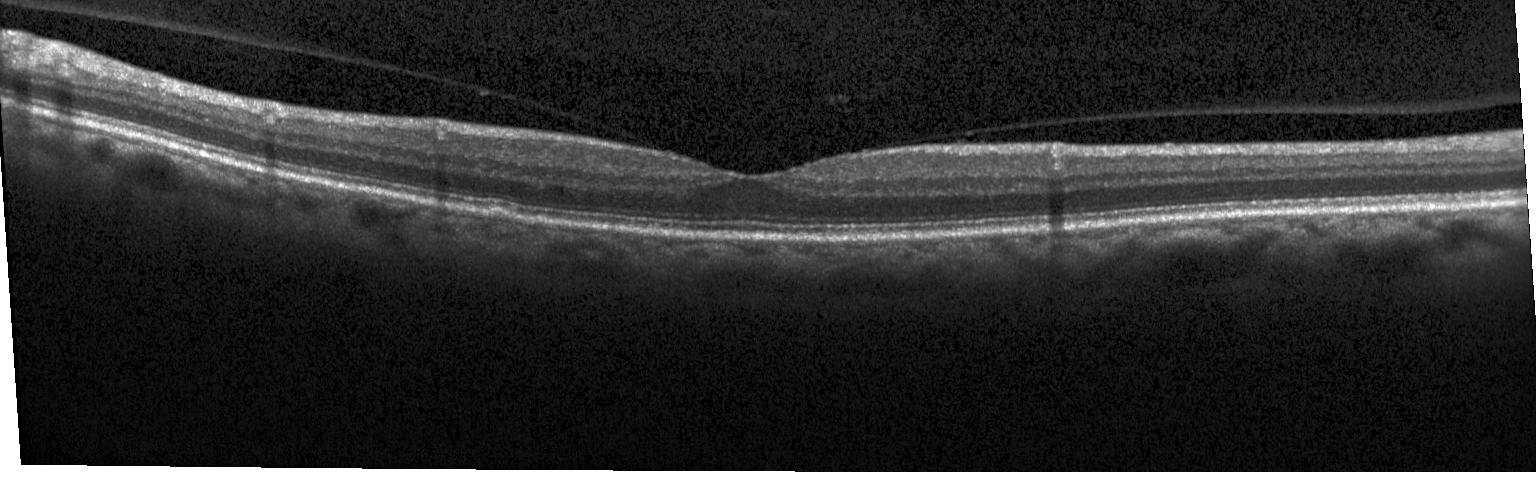
OCT line scan. Instrument: Heidelberg Spectralis. Through the macula. Spectral-domain optical coherence tomography
OCT finding: no evidence of choroidal neovascularization, diabetic macular edema, or drusen.